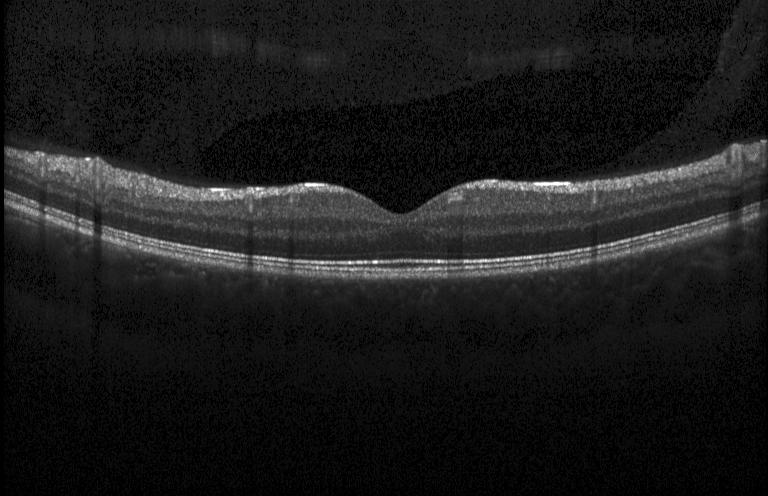
SD-OCT · OCT B-scan · through the macula — Finding: no choroidal neovascularization, no diabetic macular edema, and no drusen.